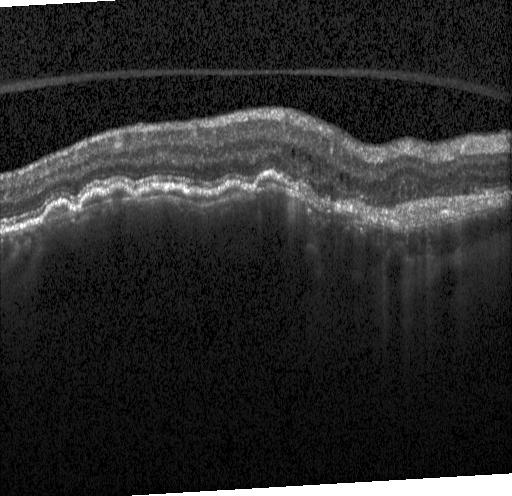
Retinal OCT cross-section. Spectral-domain optical coherence tomography. Acquired on a Heidelberg Spectralis
Finding: choroidal neovascularization (CNV).